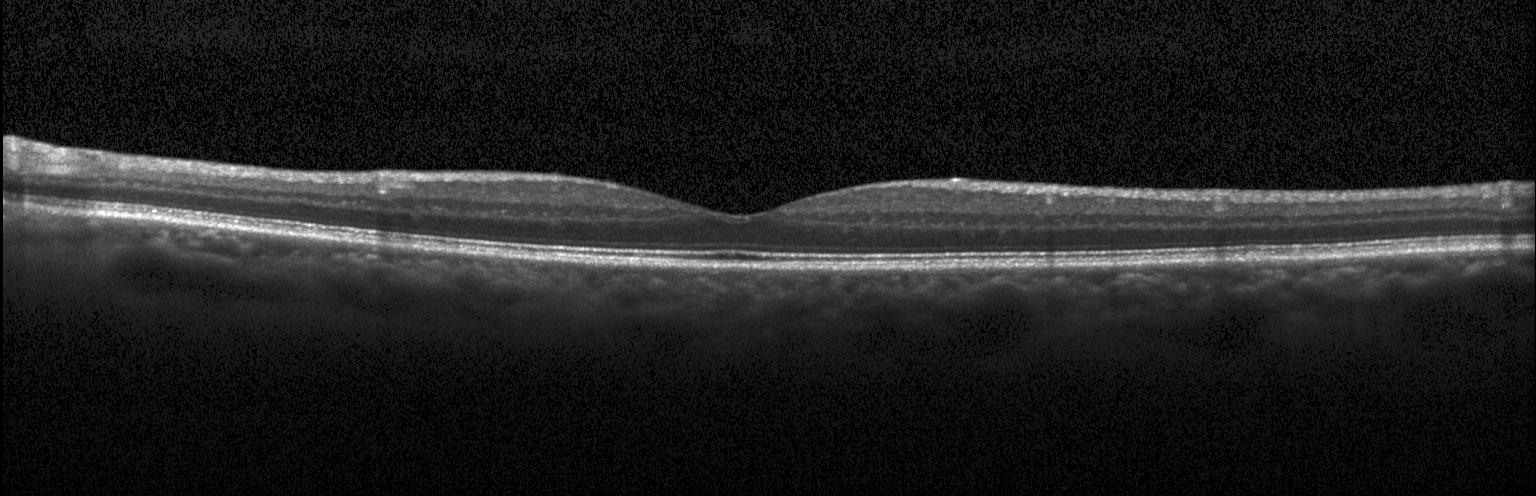

The scan shows no evidence of CNV, DME, or drusen.